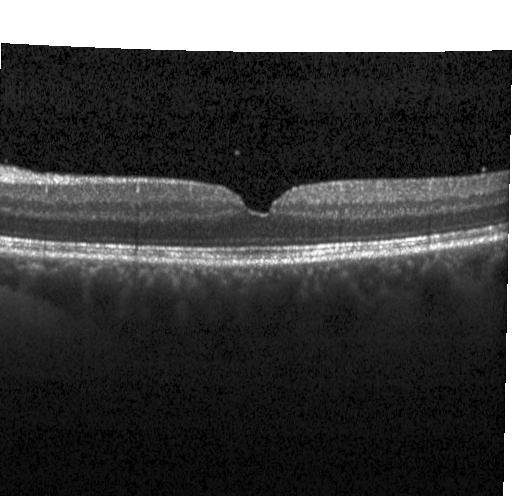 Horizontal scan through the fovea · OCT B-scan · SD-OCT · instrument: Heidelberg Spectralis — OCT finding: neither choroidal neovascularization, diabetic macular edema, nor drusen.